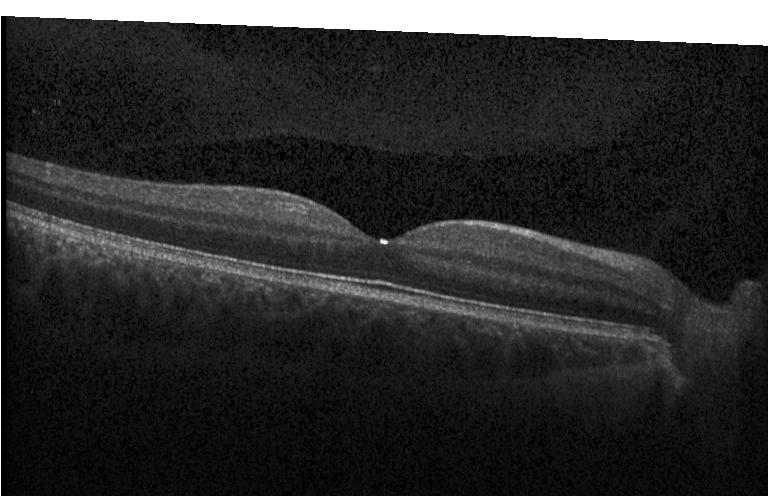

Optical coherence tomography scan. Fovea-centered — Impression: no CNV, DME, or drusen.